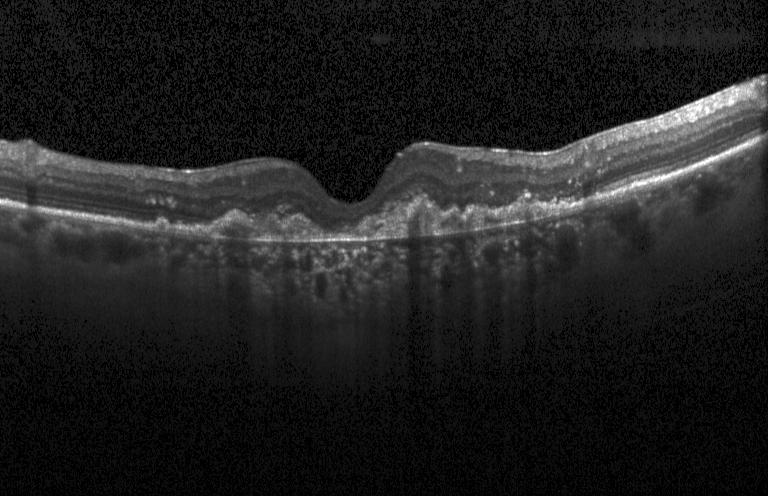
Through the macula. SD-OCT. Retinal OCT cross-section. Choroidal neovascularization.